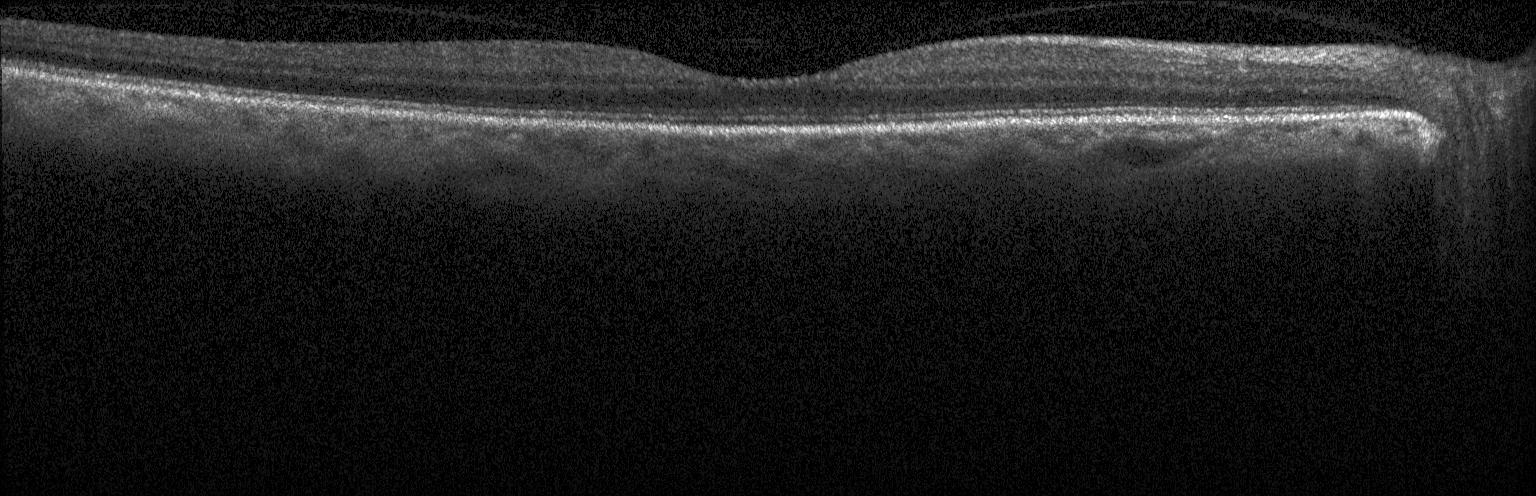

OCT scan showing no choroidal neovascularization, diabetic macular edema, or drusen.